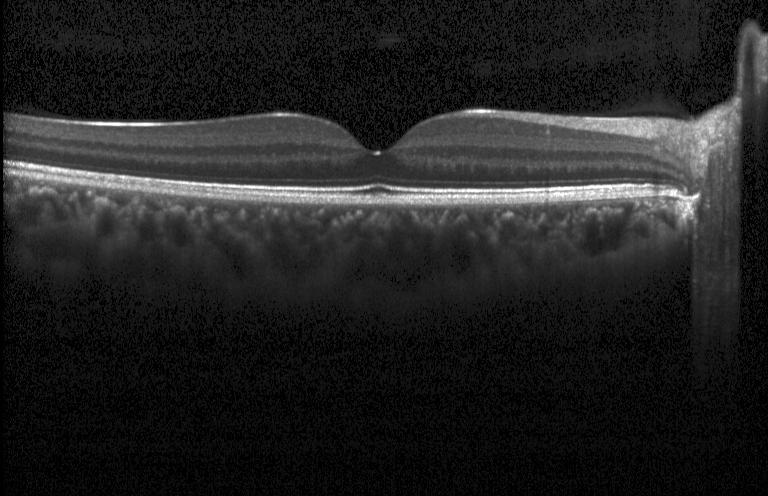
Optical coherence tomography B-scan. Spectral-domain OCT. Fovea-centered. Heidelberg Spectralis OCT system.
Finding: no choroidal neovascularization, diabetic macular edema, or drusen.